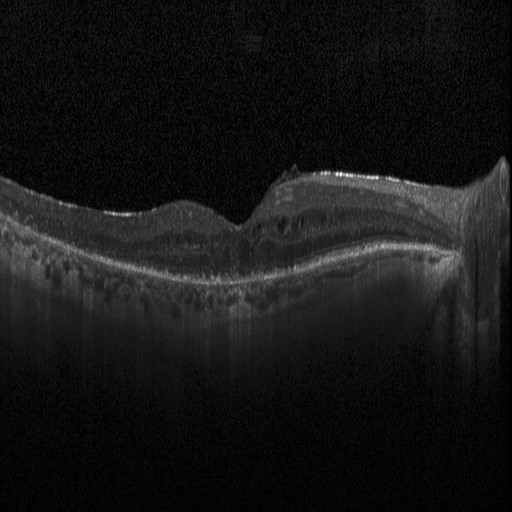
Macular scan; spectral-domain OCT; Heidelberg Spectralis OCT system; retinal OCT cross-section.
OCT finding: diabetic macular edema (DME).